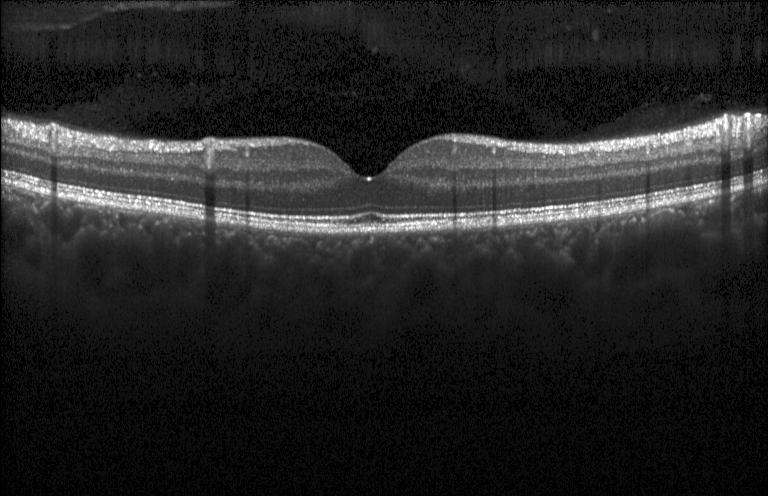
Diagnosis: no choroidal neovascularization, diabetic macular edema, or drusen.